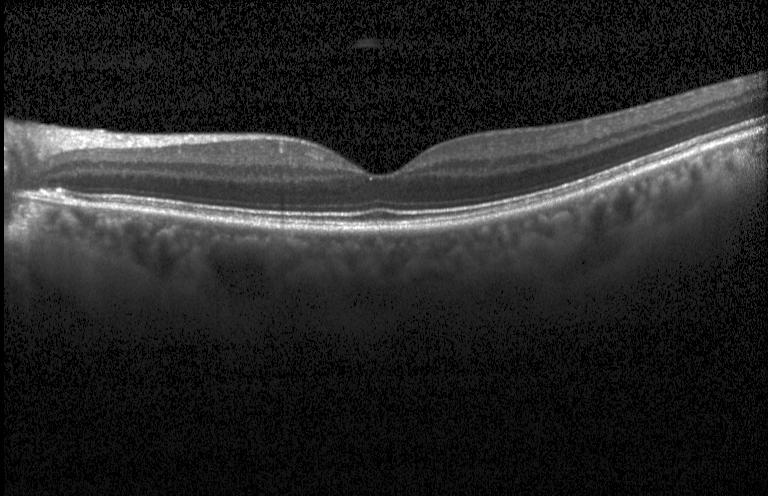 OCT B-scan. Finding: no CNV, no DME, and no drusen.